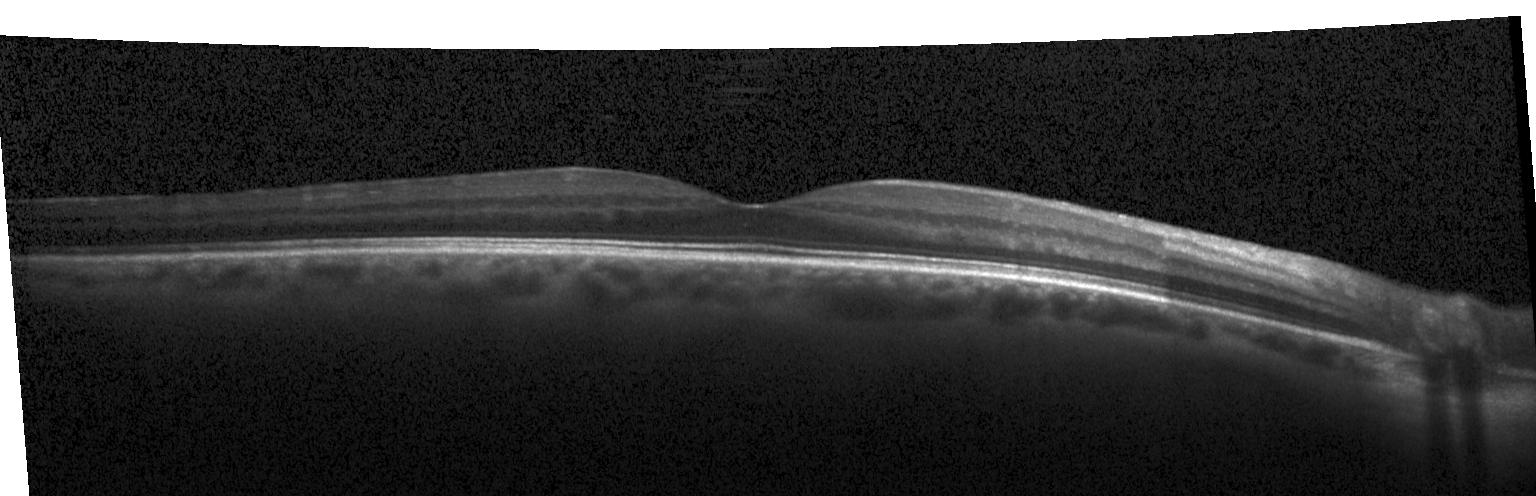 Retinal OCT cross-section. Diagnosis: no choroidal neovascularization, diabetic macular edema, or drusen.